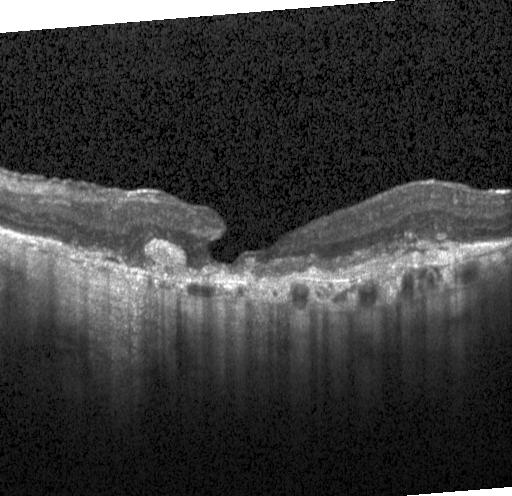 Macular OCT: a choroidal neovascular membrane.